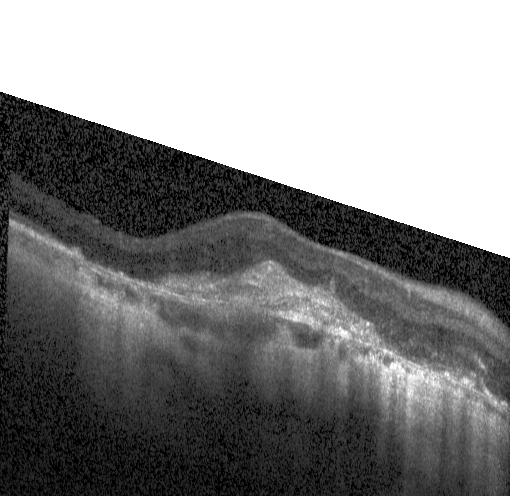
OCT scan showing choroidal neovascularization.